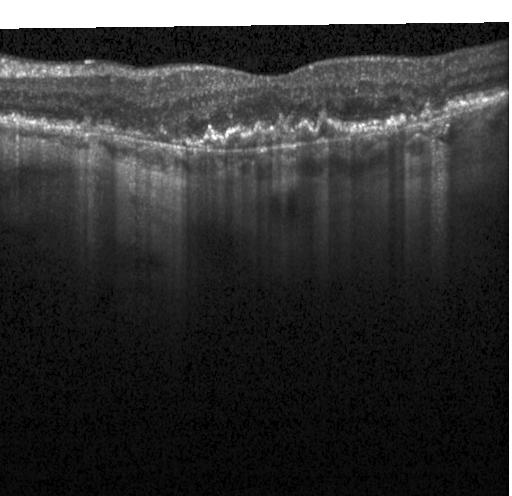
OCT scan showing choroidal neovascularization (CNV).